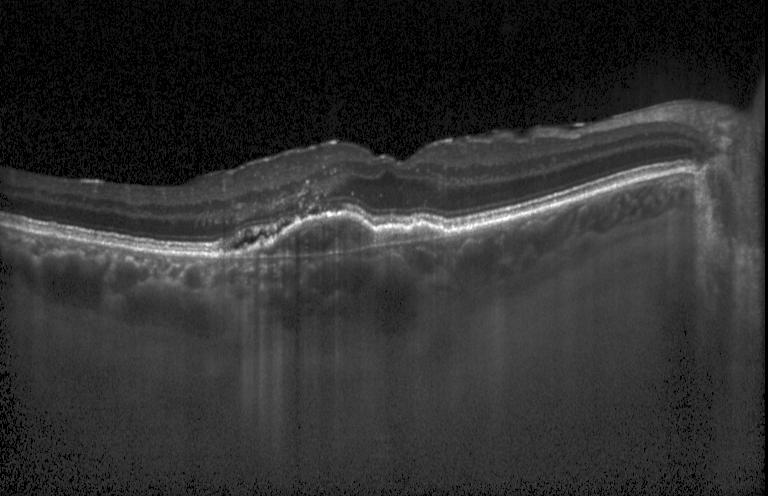
Optical coherence tomography B-scan; through the macula; SD-OCT. Diagnosis: choroidal neovascularization (CNV).